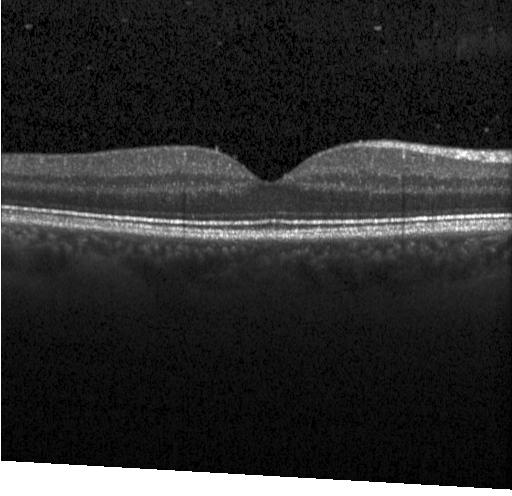 Impression: no CNV, DME, or drusen.